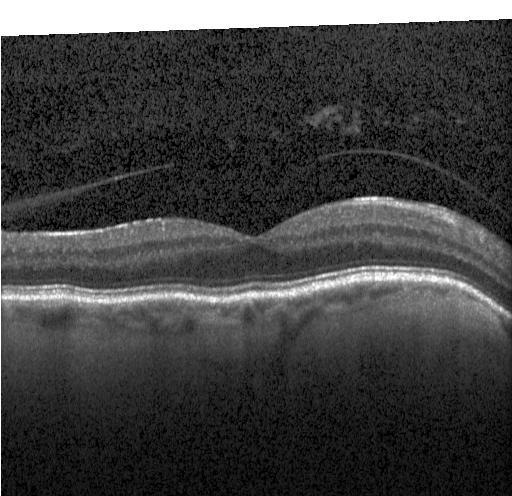 OCT finding: no choroidal neovascularization, no diabetic macular edema, and no drusen.